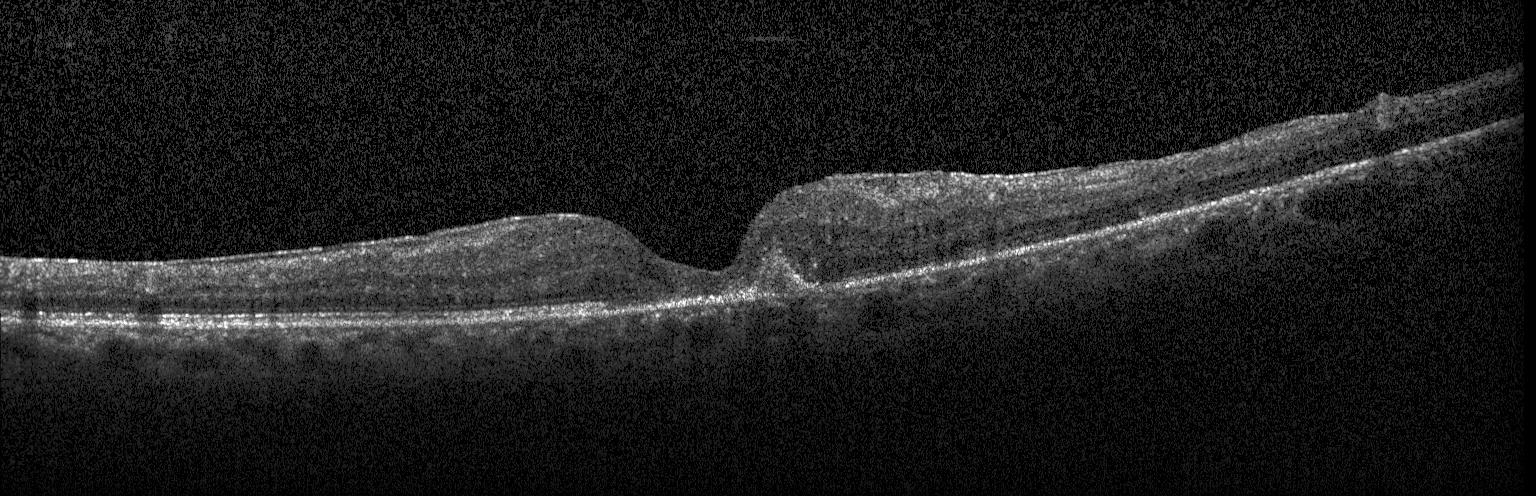

Retinal OCT B-scan.
Impression: choroidal neovascularization.